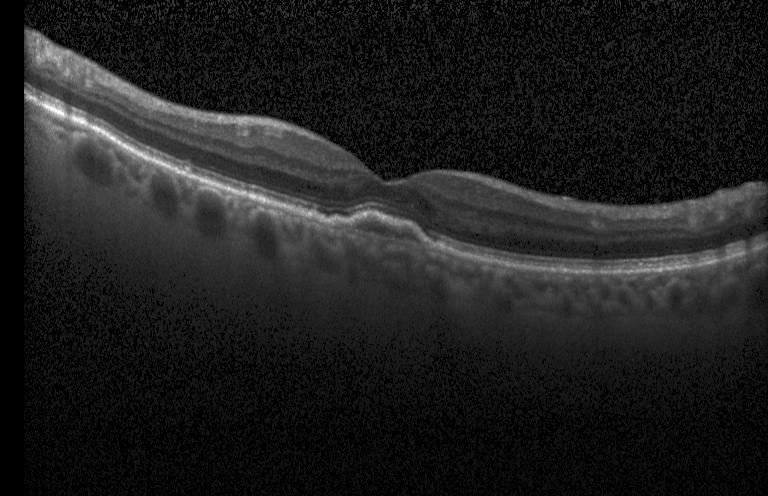 Macular OCT demonstrating a choroidal neovascular membrane.